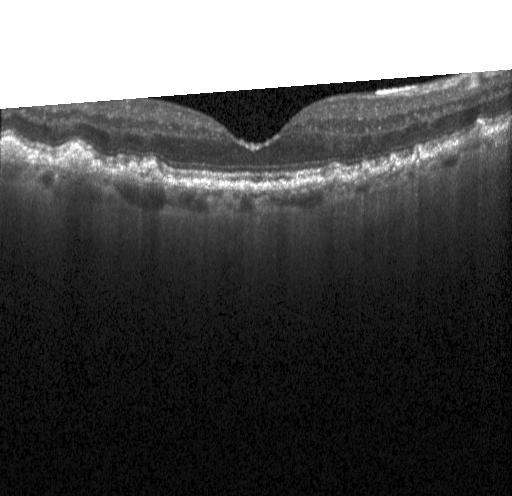 Optical coherence tomography scan
The scan shows drusen.